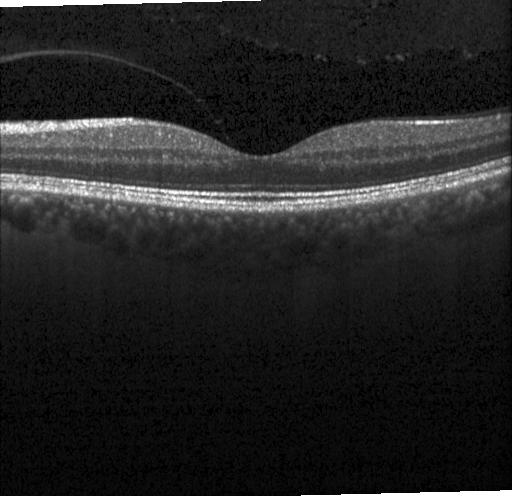 Dx: neither choroidal neovascularization, diabetic macular edema, nor drusen.